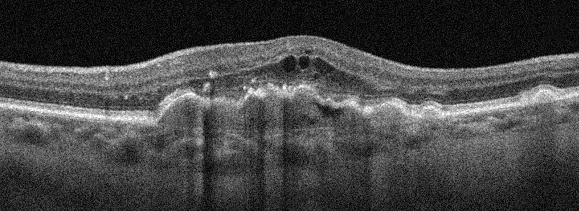

Impression: AMD.